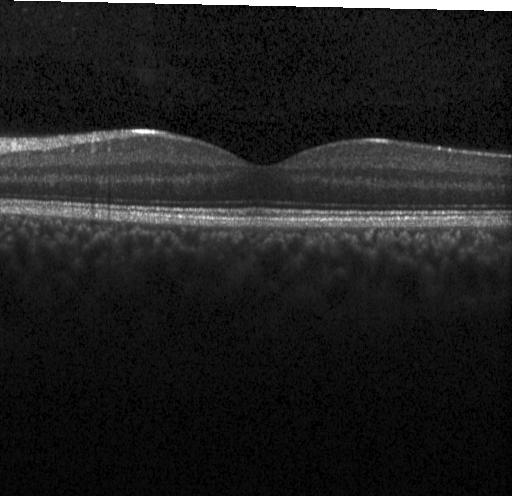 Retinal OCT cross-section — Diagnosis: neither choroidal neovascularization, diabetic macular edema, nor drusen.